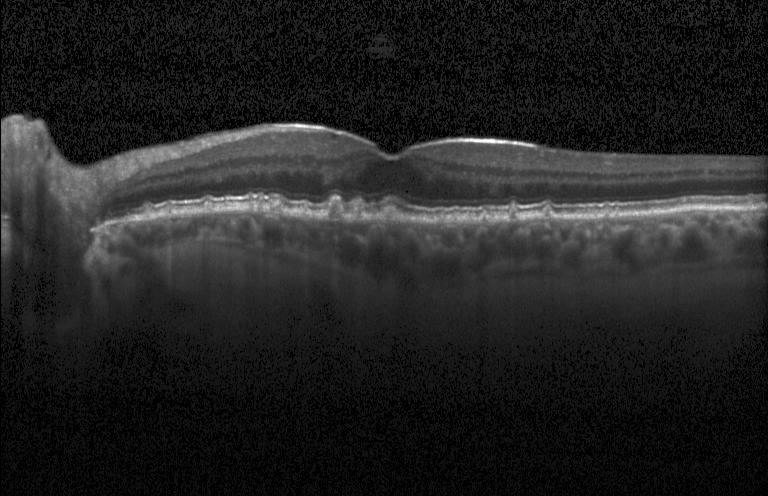
Impression: sub-RPE drusenoid deposits.